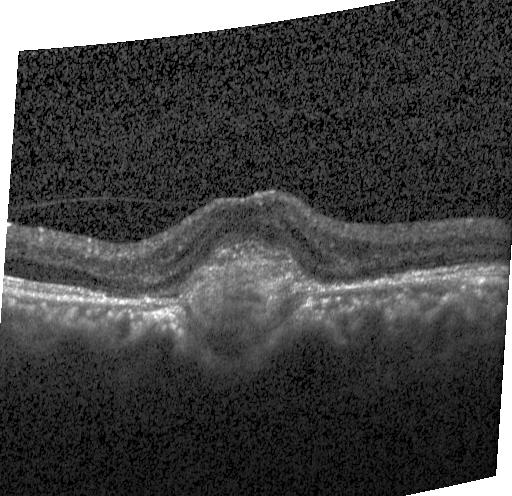

This B-scan demonstrates a choroidal neovascular membrane.